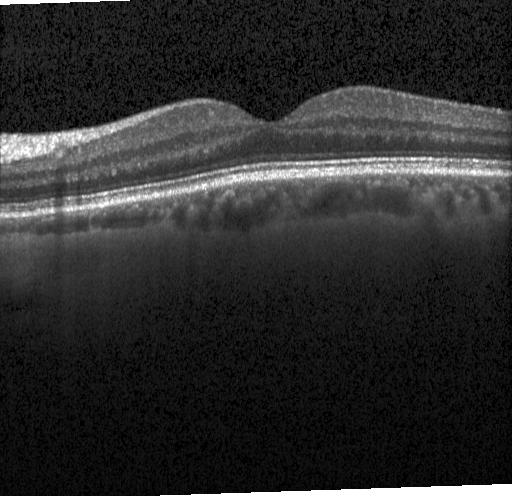
Retinal OCT B-scan. The scan shows no evidence of CNV, DME, or drusen.